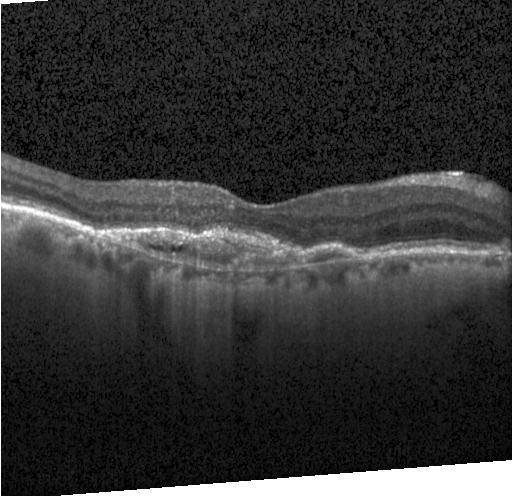 Macular scan, optical coherence tomography scan, Heidelberg Spectralis OCT system, SD-OCT.
Assessment: CNV.